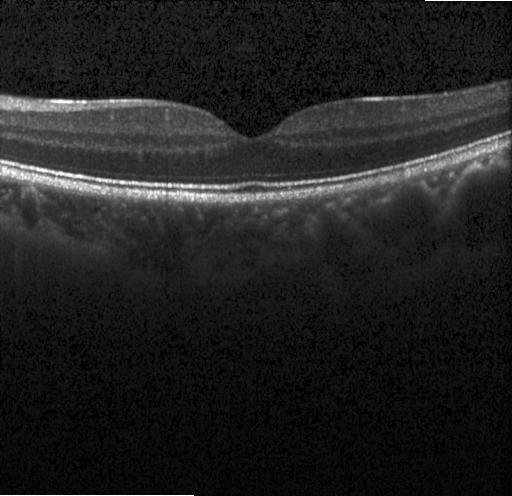
Assessment: no evidence of CNV, DME, or drusen.